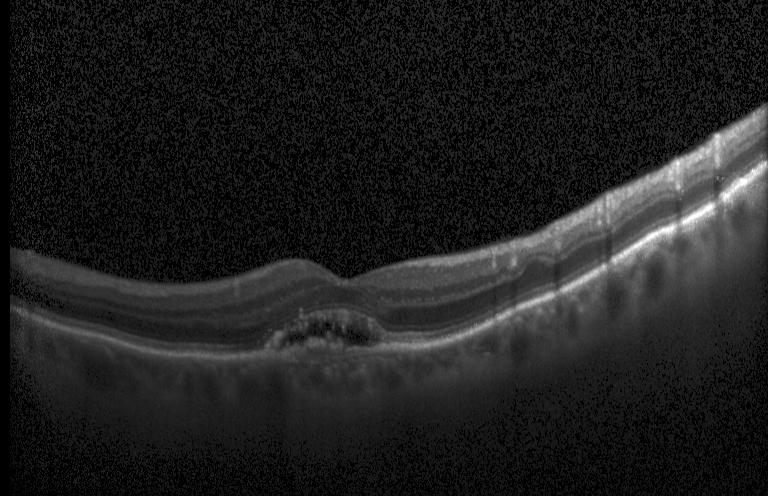

OCT B-scan showing a choroidal neovascular membrane.